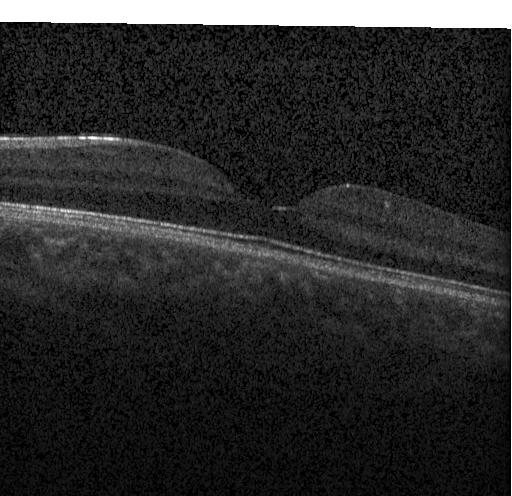 Retinal OCT B-scan · Heidelberg Spectralis · through the macula — No choroidal neovascularization, no diabetic macular edema, and no drusen.